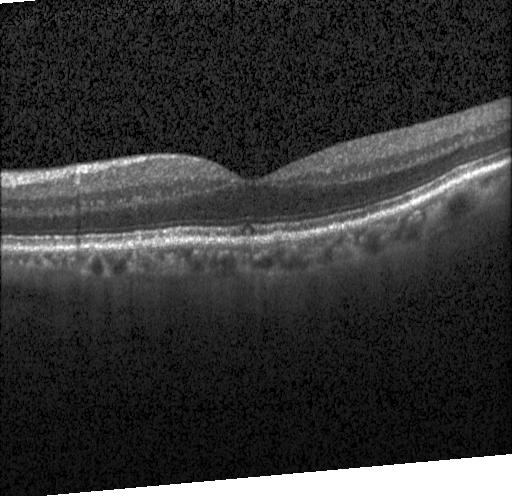

Spectral-domain OCT; OCT line scan; Heidelberg Spectralis OCT system; centered on the fovea.
Diagnosis: no evidence of choroidal neovascularization, diabetic macular edema, or drusen.